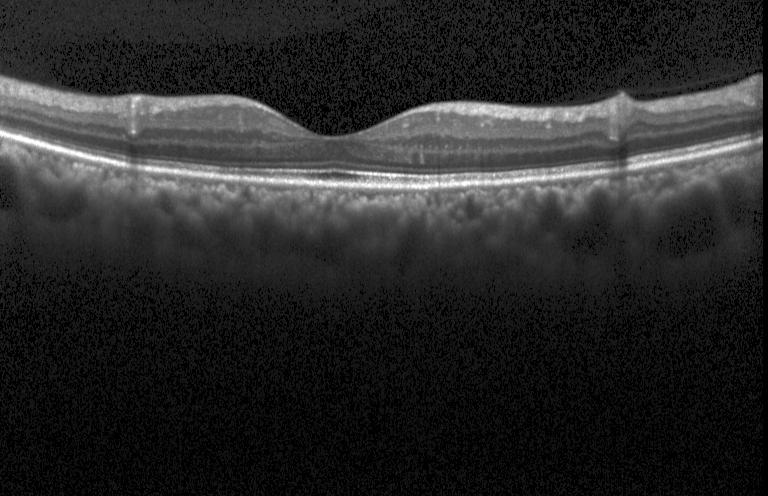 Retinal OCT B-scan. Finding: no evidence of choroidal neovascularization, diabetic macular edema, or drusen.